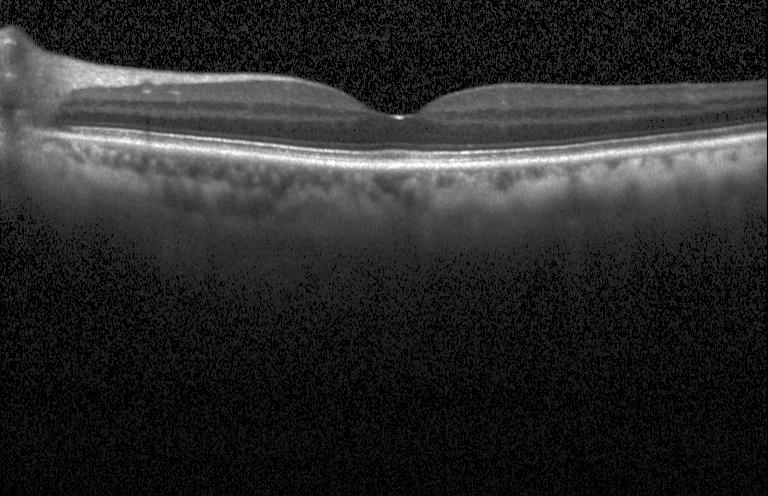 Finding: no choroidal neovascularization, diabetic macular edema, or drusen.